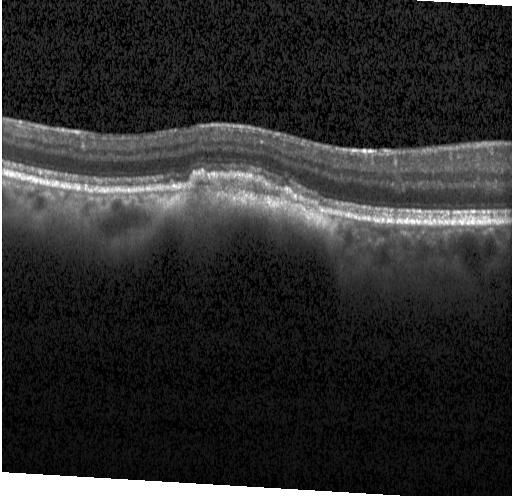 Spectral-domain optical coherence tomography · OCT line scan · Heidelberg Spectralis.
OCT finding: a choroidal neovascular membrane.